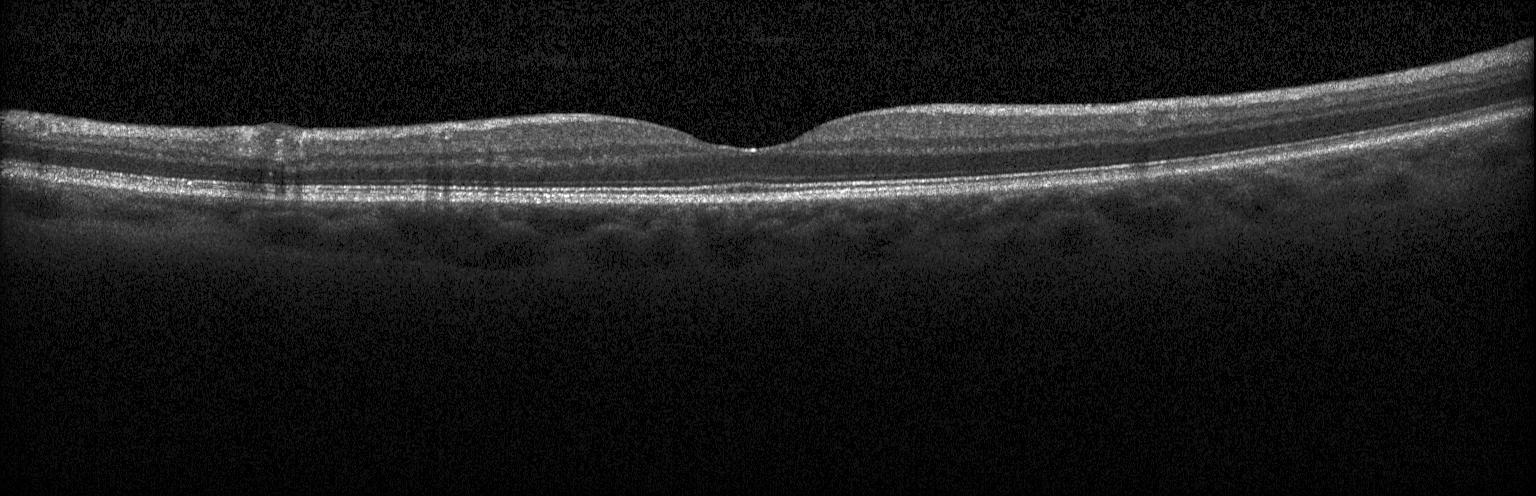
OCT B-scan
Dx: no evidence of choroidal neovascularization, diabetic macular edema, or drusen.